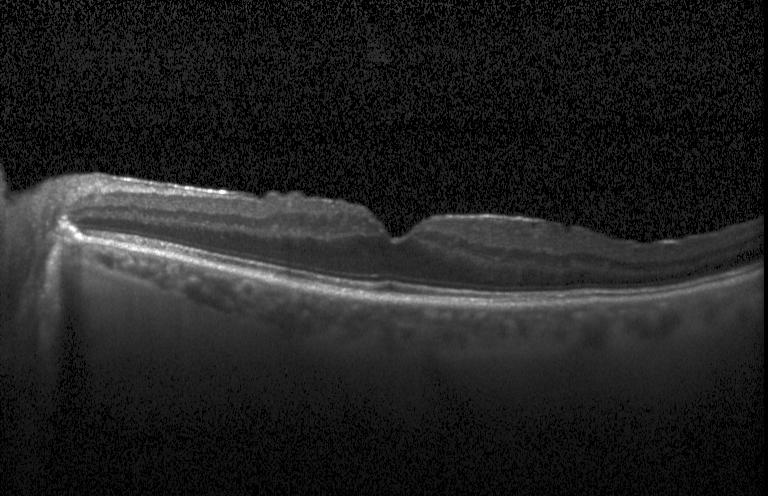
Impression: no evidence of choroidal neovascularization, diabetic macular edema, or drusen.